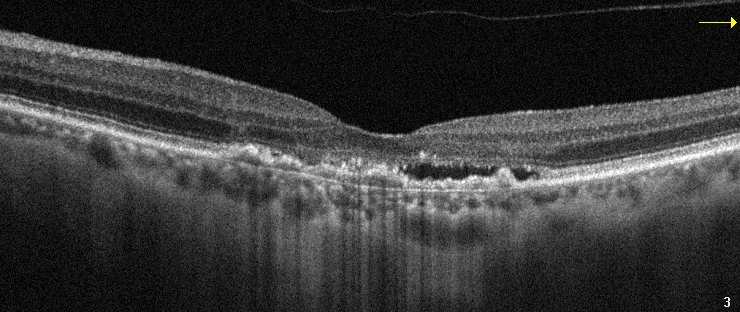

OCT B-scan.
Impression: AMD.